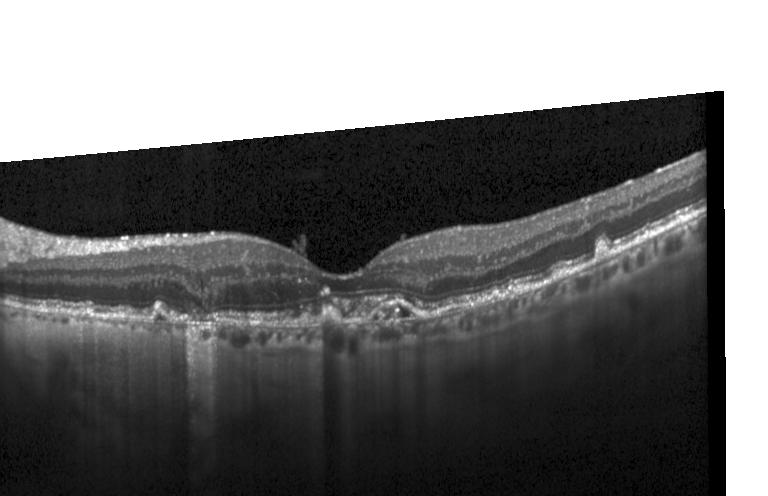 Optical coherence tomography B-scan · acquired on a Heidelberg Spectralis. Dx: choroidal neovascularization.